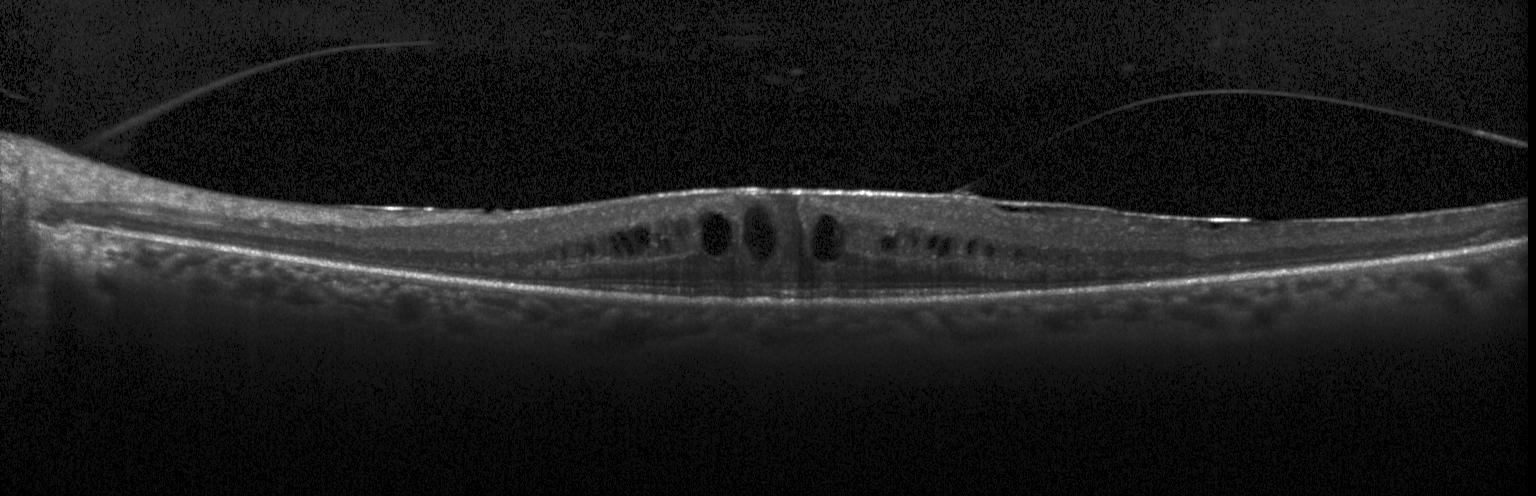 Optical coherence tomography B-scan, horizontal scan through the fovea — Finding: diabetic macular edema.